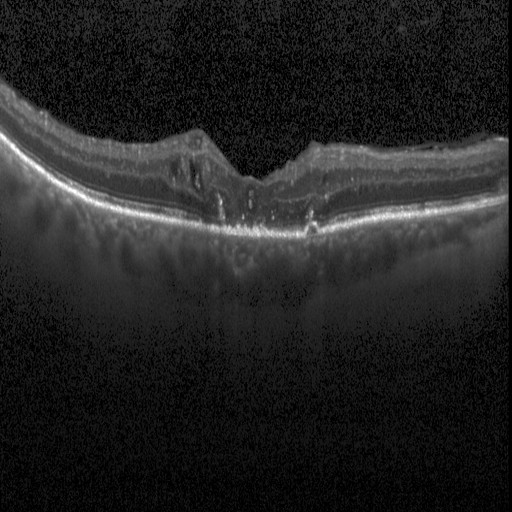

Finding: diabetic macular edema.